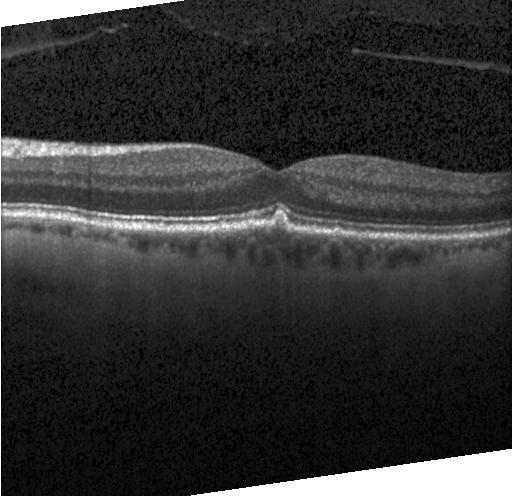
Diagnosis: multiple drusen.